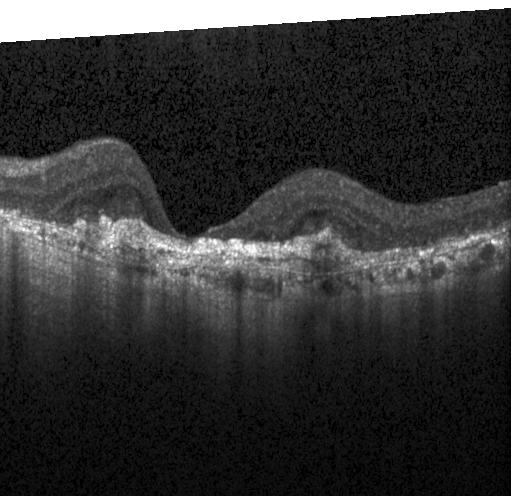

Instrument: Heidelberg Spectralis. Optical coherence tomography B-scan
Finding: choroidal neovascularization (CNV).